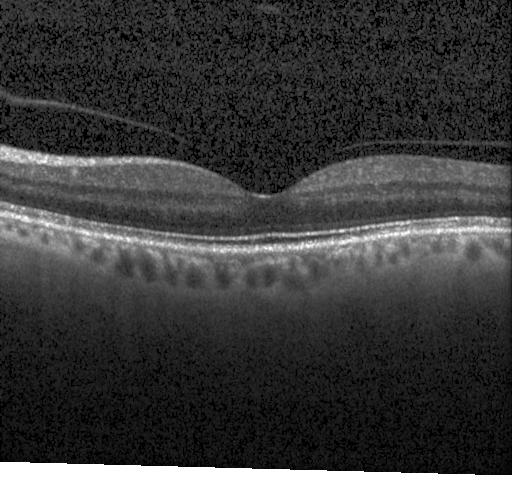 Diagnosis: neither choroidal neovascularization, diabetic macular edema, nor drusen.